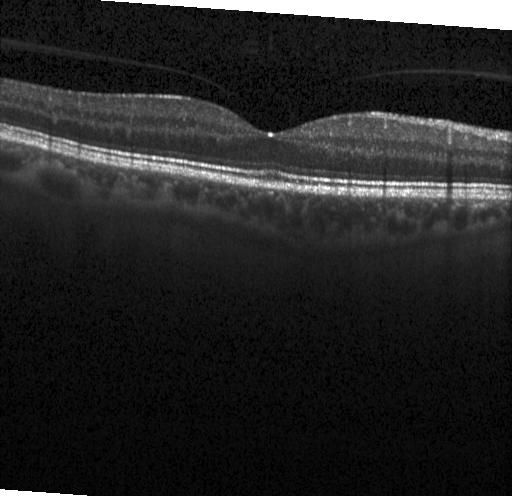 Optical coherence tomography scan
Diagnosis: no choroidal neovascularization, diabetic macular edema, or drusen.